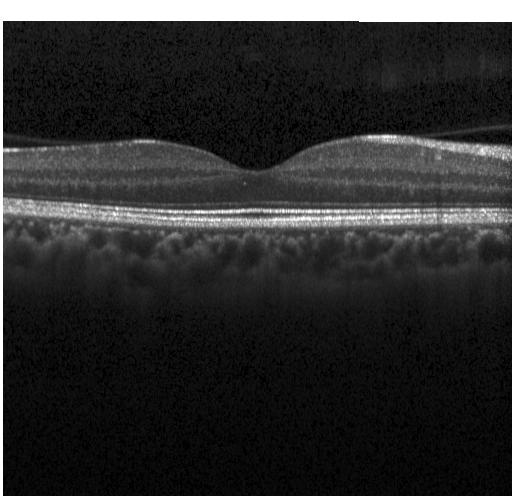

Retinal OCT cross-section.
Impression: neither CNV, DME, nor drusen.